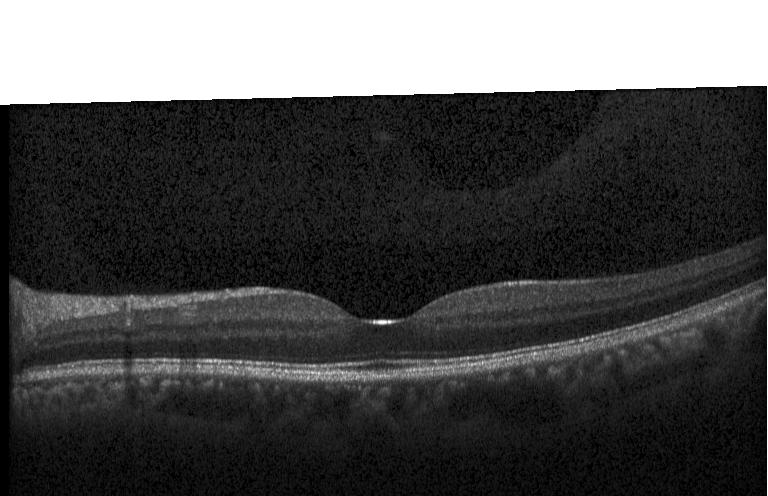
Finding: no choroidal neovascularization, diabetic macular edema, or drusen.